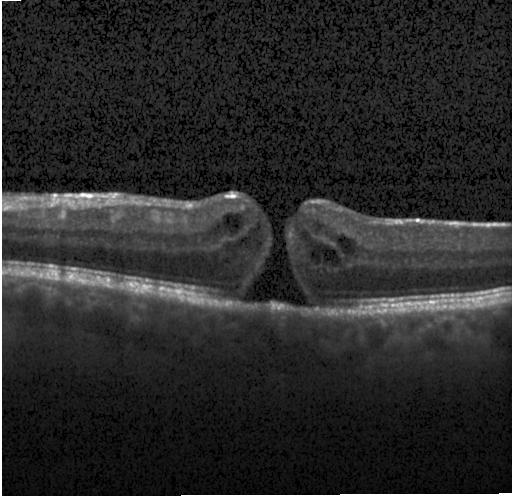

Optical coherence tomography scan · Heidelberg Spectralis OCT system. Finding: diabetic macular edema (DME).